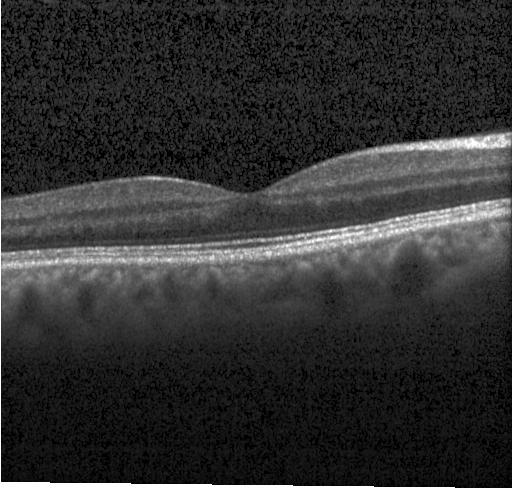 Fovea-centered, optical coherence tomography B-scan, spectral-domain optical coherence tomography. Finding: no CNV, DME, or drusen.